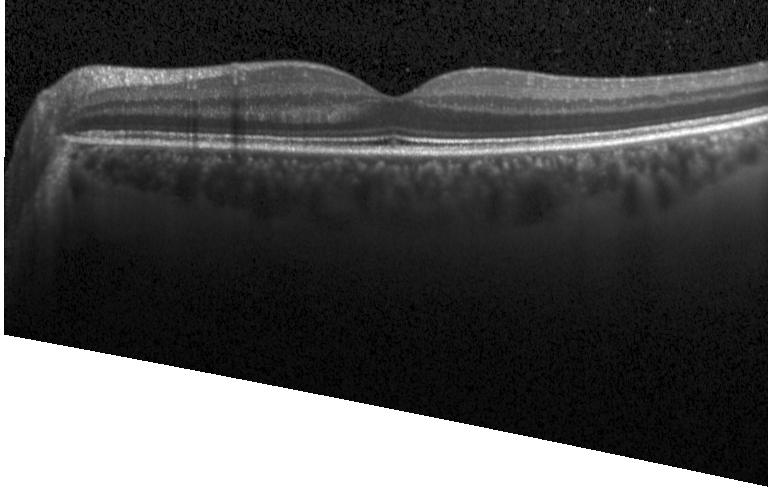

Retinal OCT B-scan, spectral-domain optical coherence tomography
Impression: no CNV, DME, or drusen.